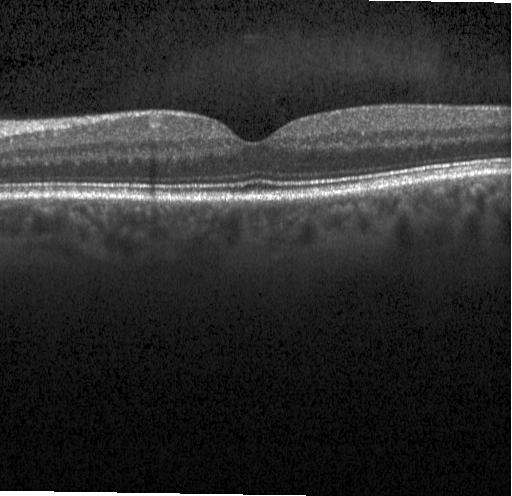
Diagnosis: neither choroidal neovascularization, diabetic macular edema, nor drusen.